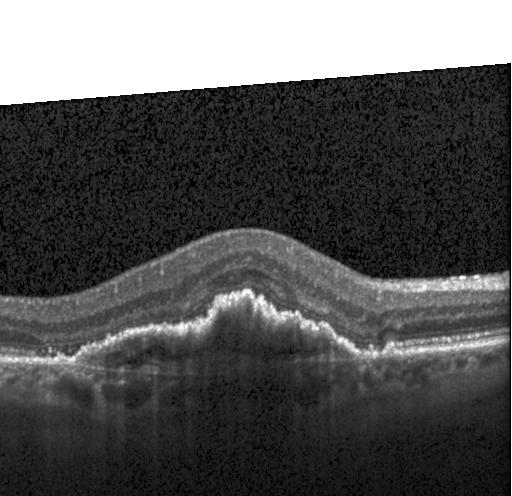
Horizontal scan through the fovea; Heidelberg Spectralis; optical coherence tomography B-scan; spectral-domain OCT — Finding: a choroidal neovascular membrane.